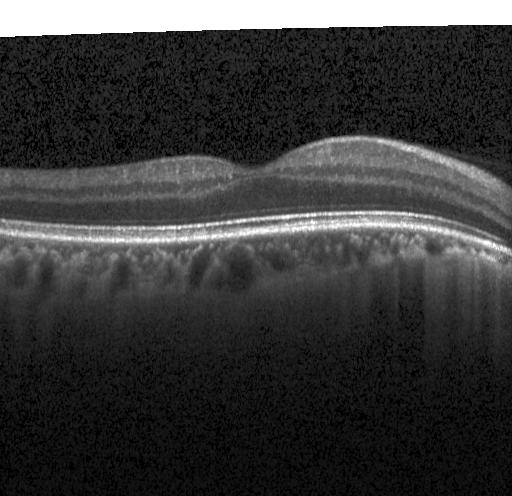 Instrument: Heidelberg Spectralis, retinal OCT cross-section. Diagnosis: no choroidal neovascularization, no diabetic macular edema, and no drusen.